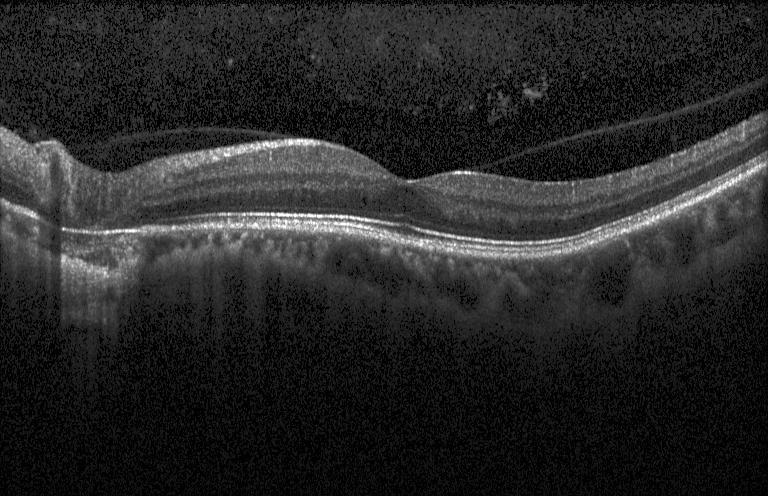

Heidelberg Spectralis. SD-OCT. Fovea-centered. OCT line scan
Diagnosis: neither choroidal neovascularization, diabetic macular edema, nor drusen.